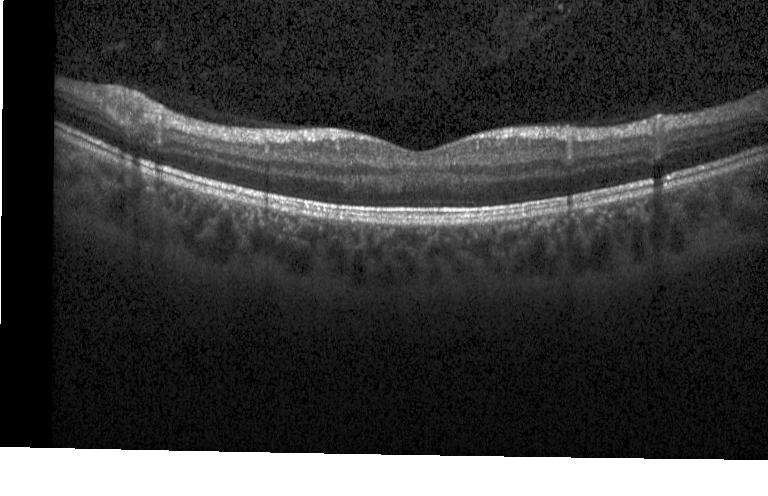
OCT scan showing no evidence of choroidal neovascularization, diabetic macular edema, or drusen.